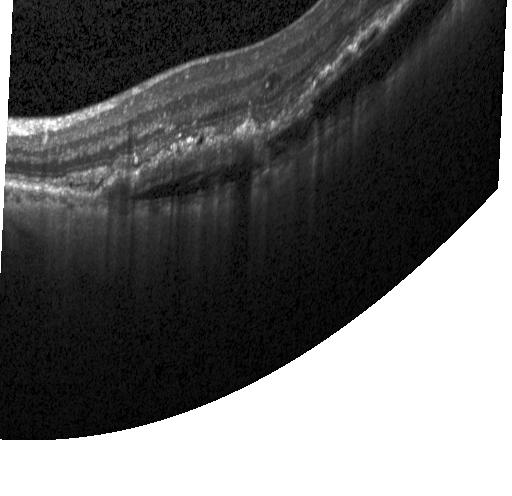 The scan shows CNV.